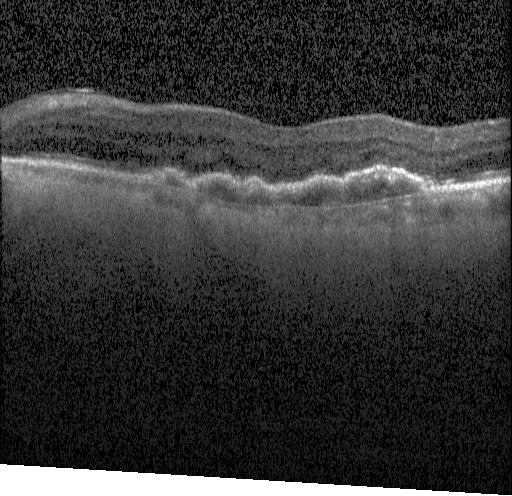
Finding: choroidal neovascularization.